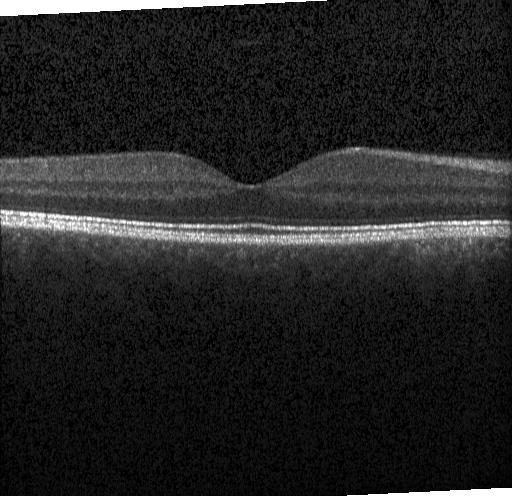 Horizontal scan through the fovea; spectral-domain OCT; Heidelberg Spectralis OCT system; optical coherence tomography B-scan
Macular OCT: neither choroidal neovascularization, diabetic macular edema, nor drusen.